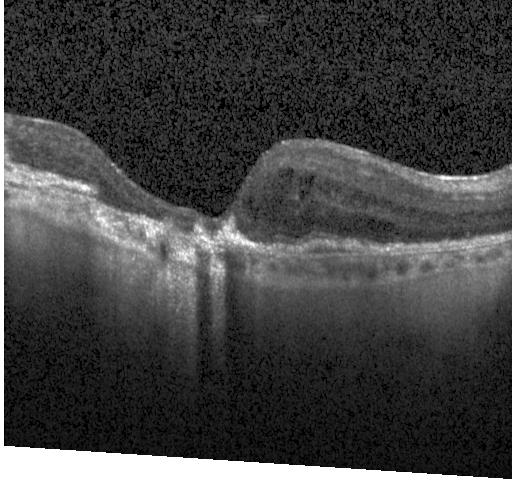
OCT scan showing choroidal neovascularization (CNV).